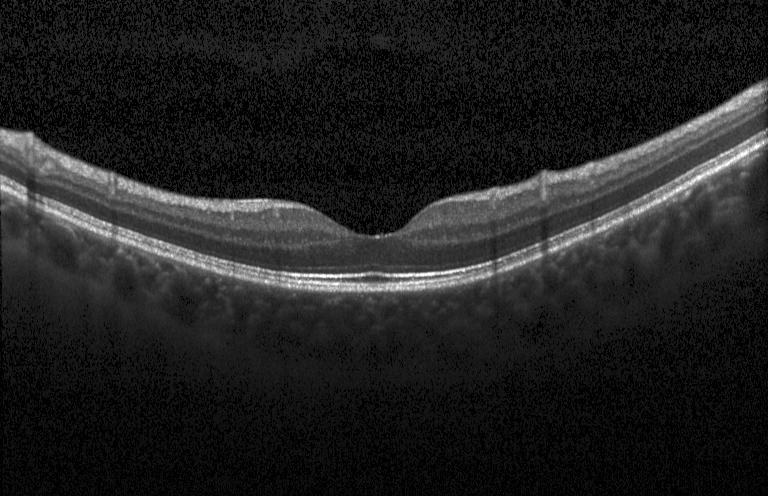 OCT line scan
Diagnosis: neither CNV, DME, nor drusen.